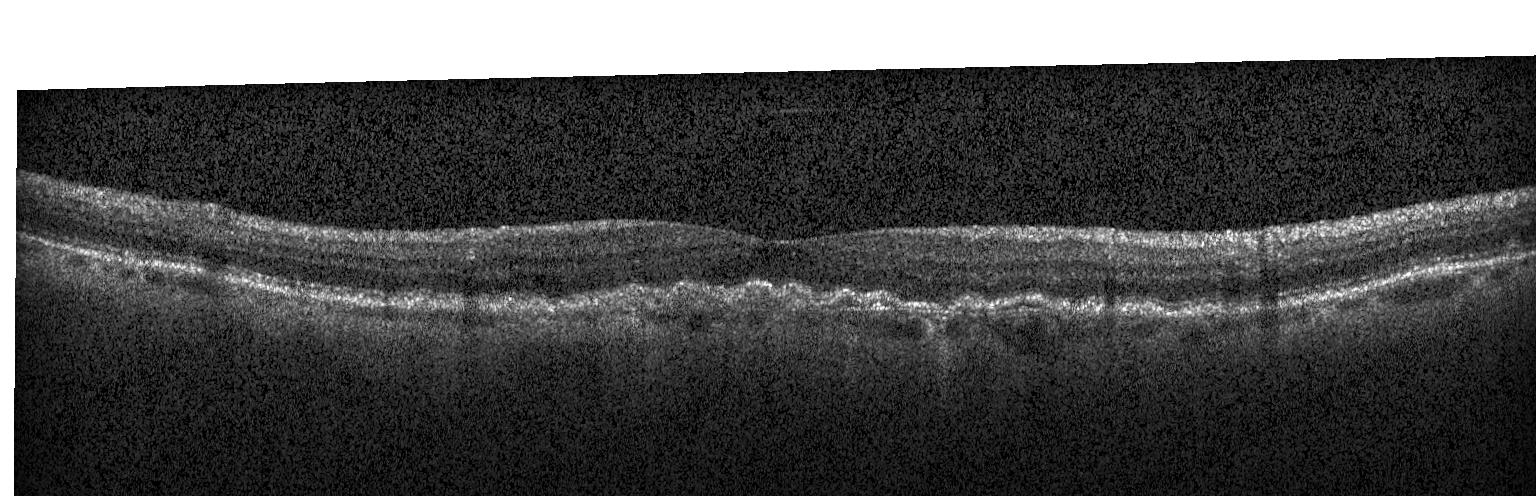
Spectral-domain OCT B-scan: a choroidal neovascular membrane.